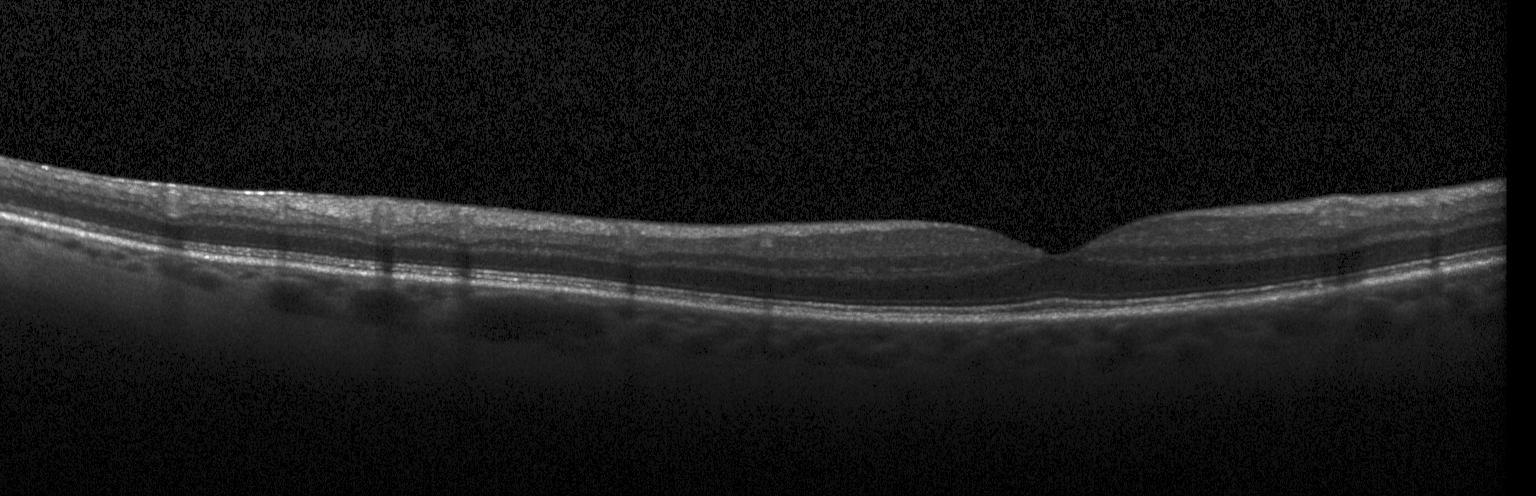
The scan shows no CNV, DME, or drusen.